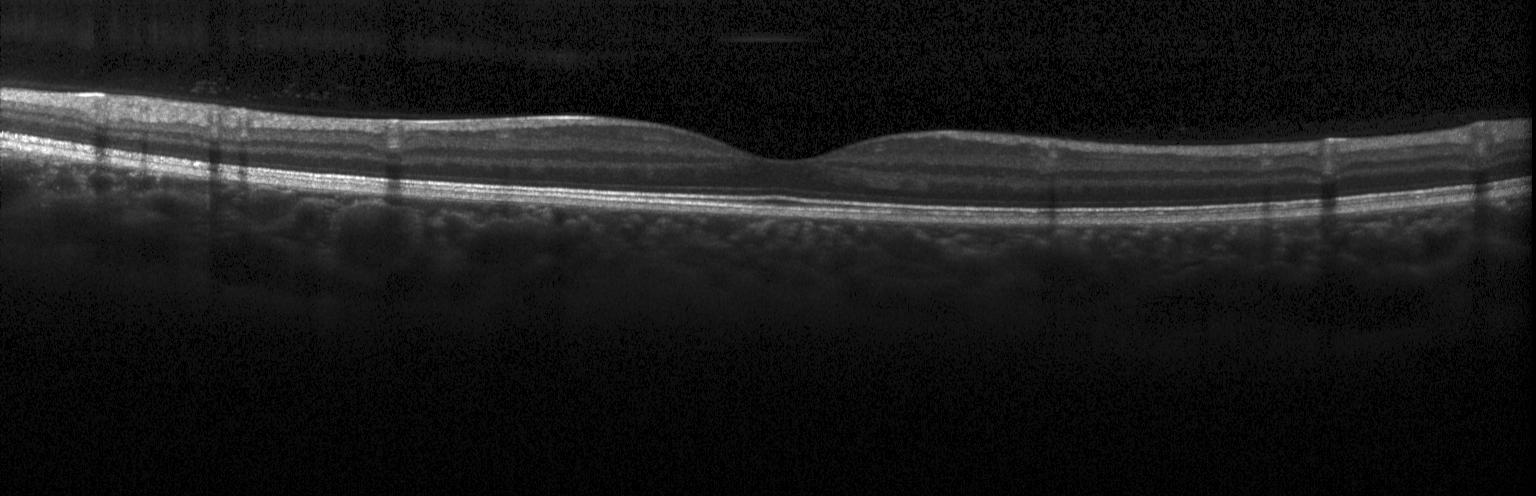 Optical coherence tomography scan · spectral-domain optical coherence tomography · Heidelberg Spectralis OCT system · centered on the fovea.
Finding: no choroidal neovascularization, diabetic macular edema, or drusen.